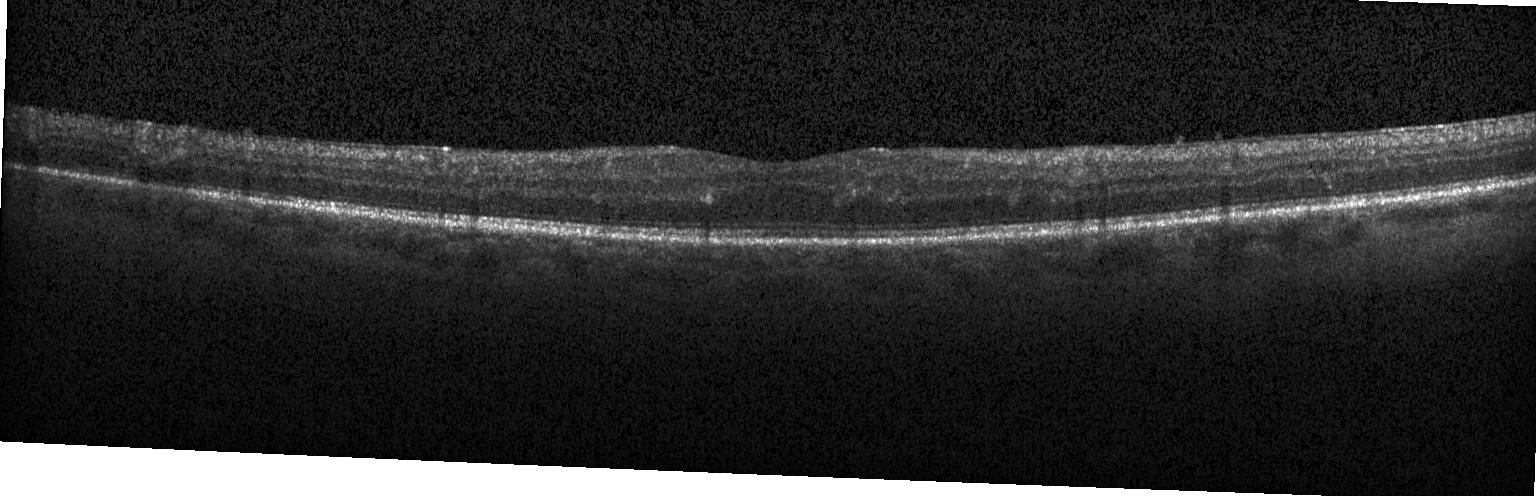
Optical coherence tomography scan; centered on the fovea; acquired on a Heidelberg Spectralis — This B-scan demonstrates no choroidal neovascularization, diabetic macular edema, or drusen.